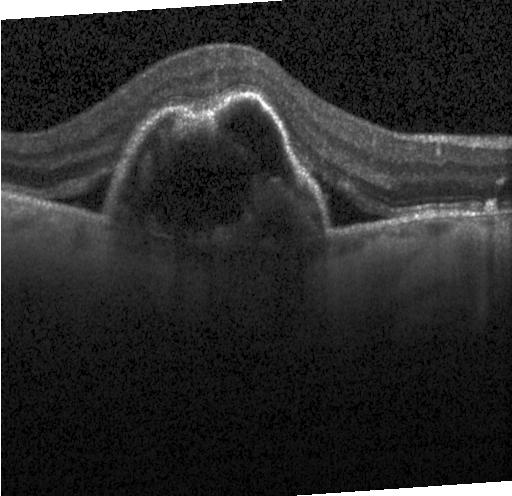

OCT finding: a choroidal neovascular membrane.